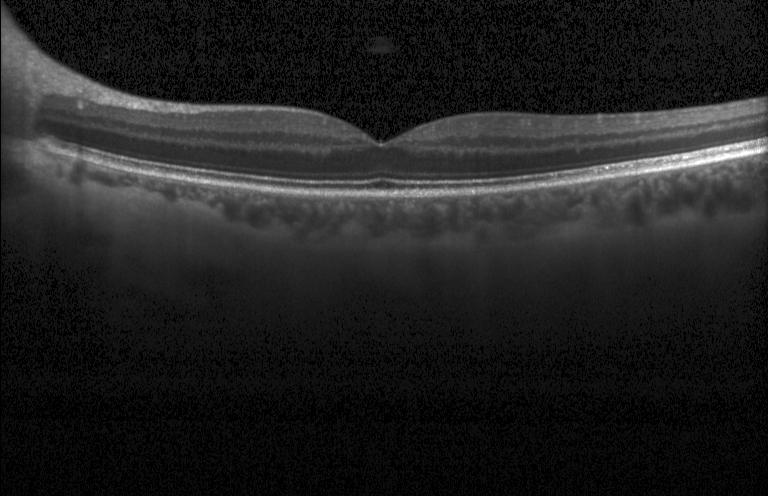 Impression: no choroidal neovascularization, diabetic macular edema, or drusen.